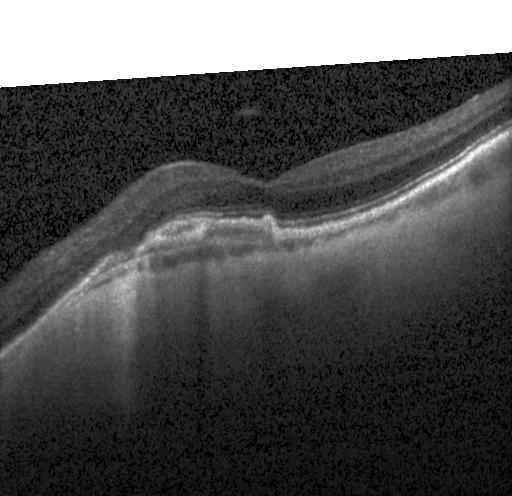

Centered on the fovea. Instrument: Heidelberg Spectralis. Retinal OCT B-scan
This B-scan demonstrates a choroidal neovascular membrane.